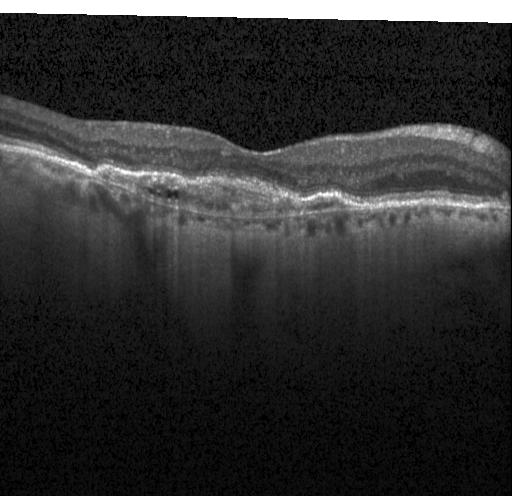

Horizontal scan through the fovea; instrument: Heidelberg Spectralis; retinal OCT cross-section; spectral-domain OCT. Diagnosis: choroidal neovascularization (CNV).